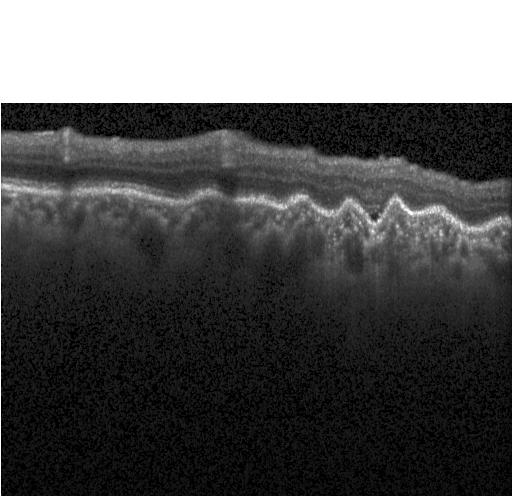

Finding: a choroidal neovascular membrane.